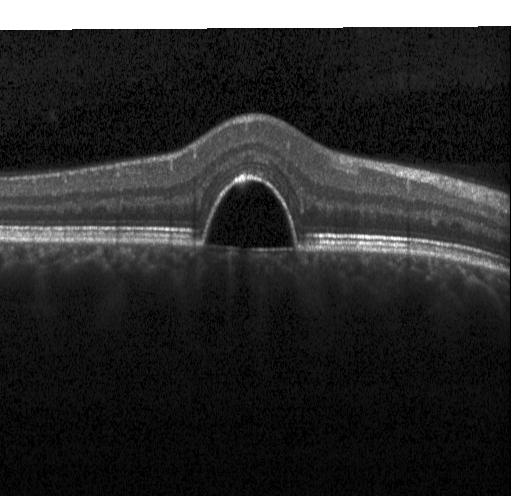
Impression: choroidal neovascularization (CNV).